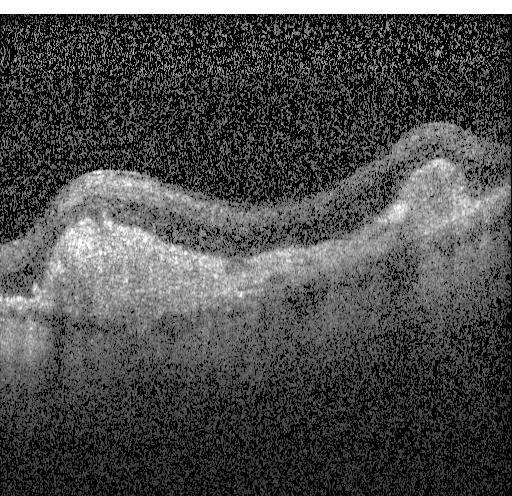
Impression: a choroidal neovascular membrane.